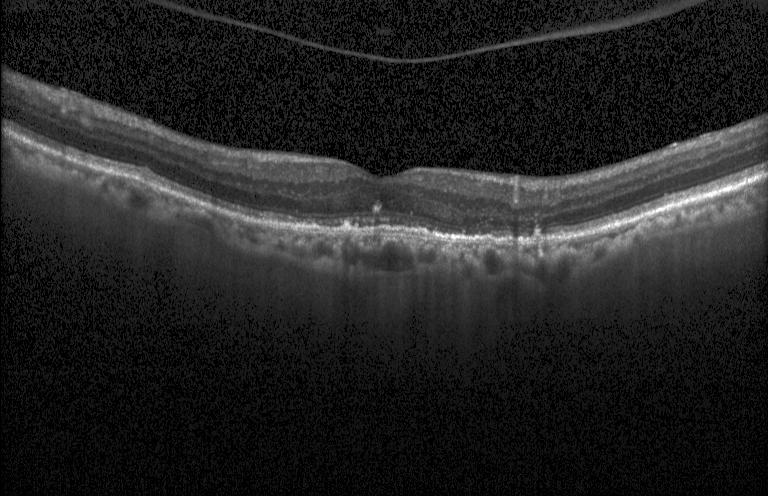
Retinal OCT cross-section showing a choroidal neovascular membrane.